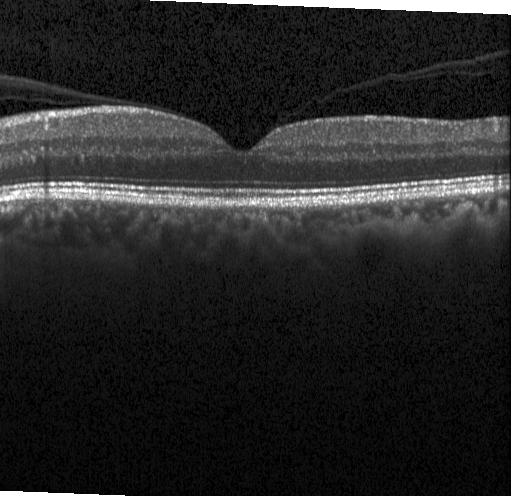

Heidelberg Spectralis OCT system; retinal OCT B-scan — OCT finding: no choroidal neovascularization, diabetic macular edema, or drusen.